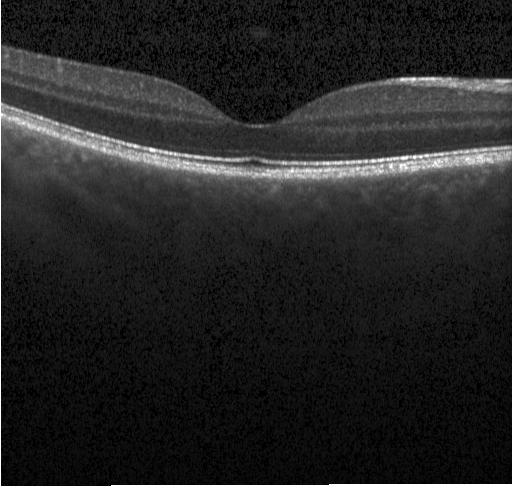

Retinal OCT B-scan
No choroidal neovascularization, no diabetic macular edema, and no drusen.